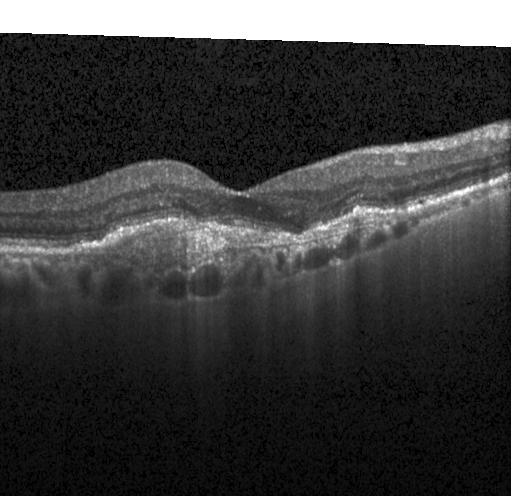
The scan shows CNV.